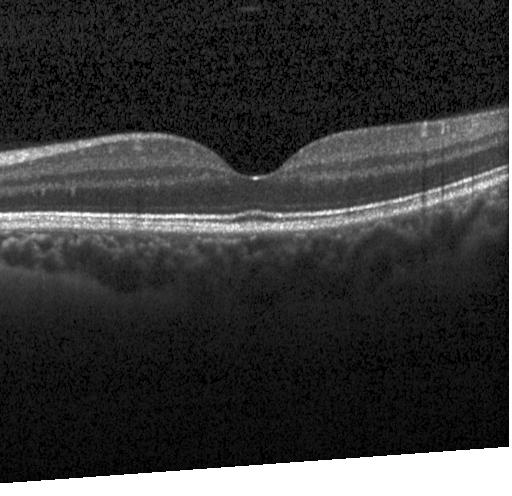
Spectral-domain optical coherence tomography, macular scan, Heidelberg Spectralis OCT system, OCT B-scan.
Impression: no CNV, no DME, and no drusen.